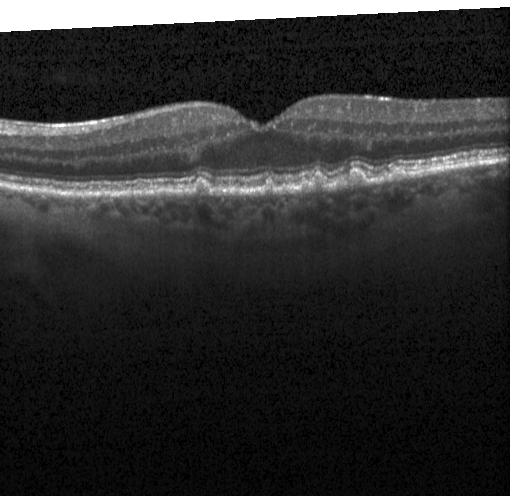

Horizontal scan through the fovea; Heidelberg Spectralis OCT system; SD-OCT; optical coherence tomography B-scan — This B-scan demonstrates multiple drusen.